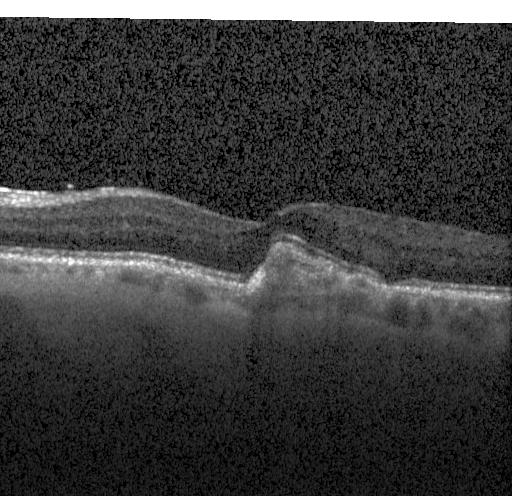 Assessment: a choroidal neovascular membrane.